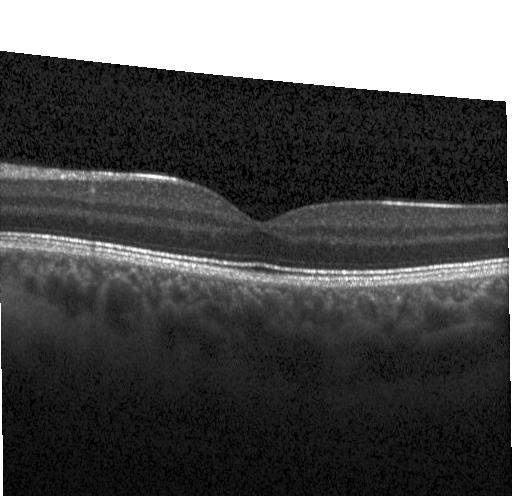

OCT finding: no CNV, no DME, and no drusen.